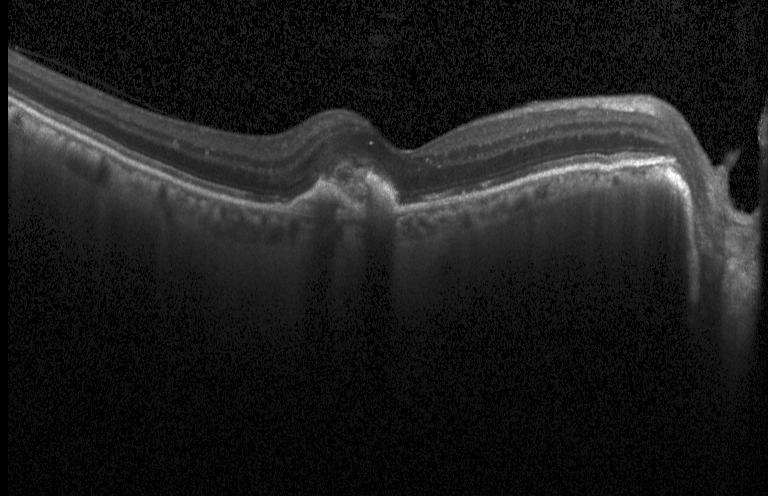
OCT line scan. Instrument: Heidelberg Spectralis. Impression: CNV.